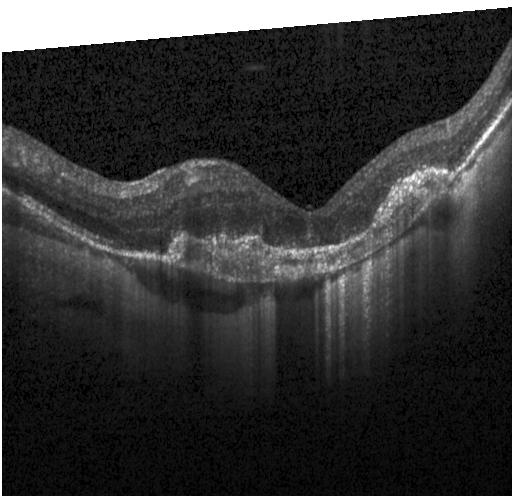

Finding: CNV.